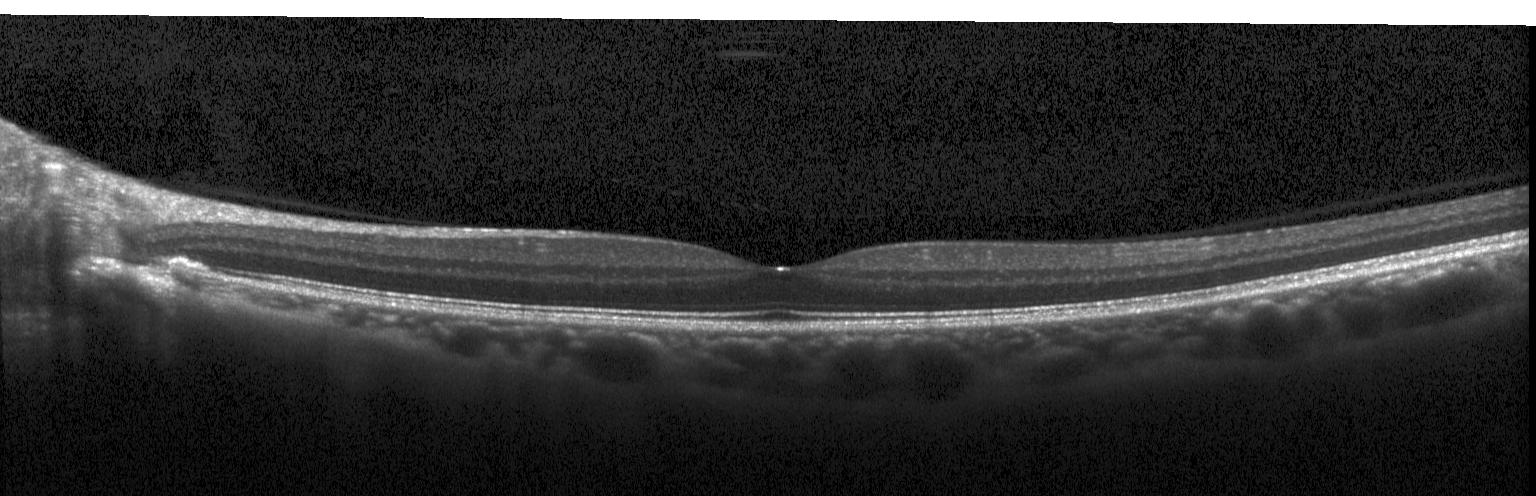 This B-scan demonstrates no choroidal neovascularization, diabetic macular edema, or drusen.